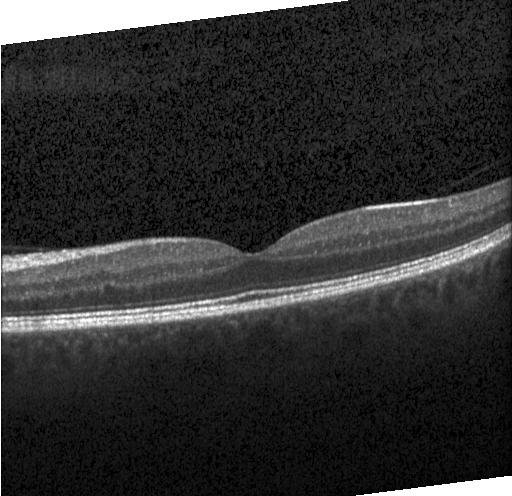
Diagnosis: no evidence of CNV, DME, or drusen.